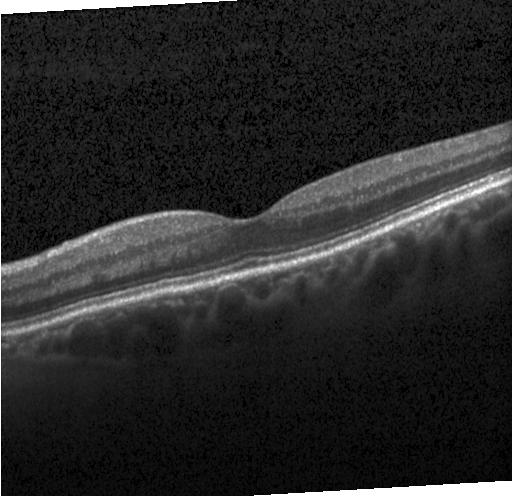 Heidelberg Spectralis OCT system · SD-OCT · through the macula · OCT B-scan. Impression: no choroidal neovascularization, diabetic macular edema, or drusen.